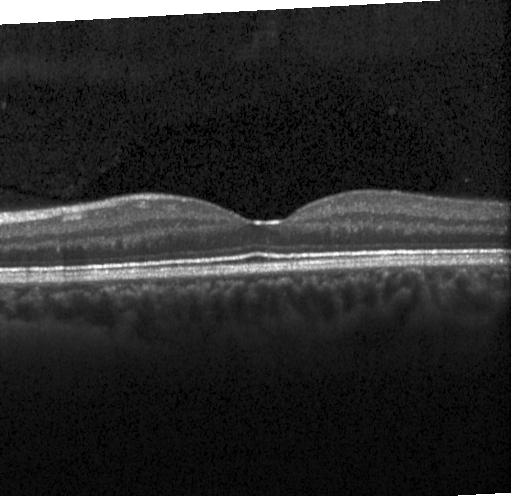
Impression: no choroidal neovascularization, diabetic macular edema, or drusen.